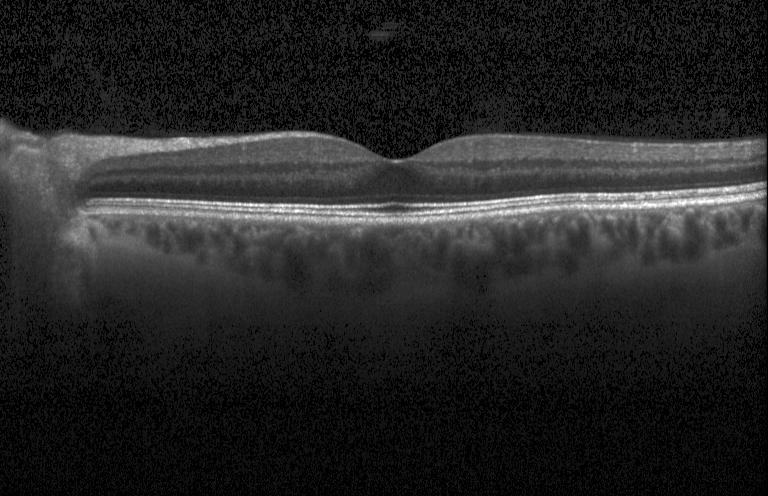 OCT B-scan showing no evidence of choroidal neovascularization, diabetic macular edema, or drusen.